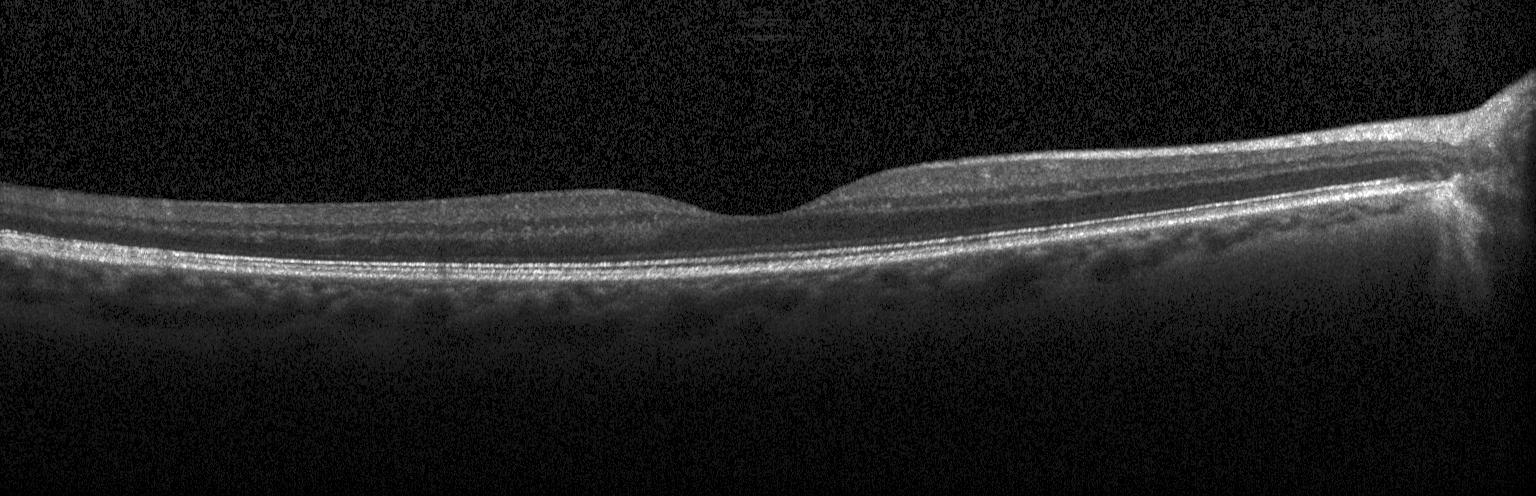

Retinal OCT cross-section, instrument: Heidelberg Spectralis, centered on the fovea — No choroidal neovascularization, diabetic macular edema, or drusen.